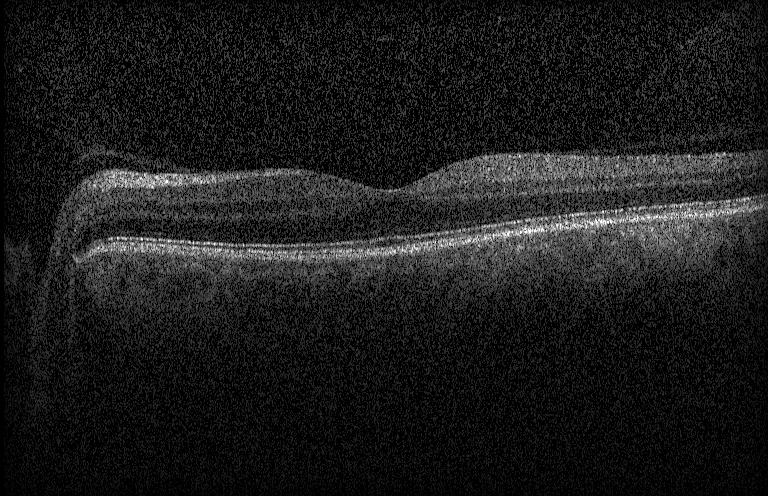
Acquired on a Heidelberg Spectralis, retinal OCT B-scan — Impression: neither CNV, DME, nor drusen.